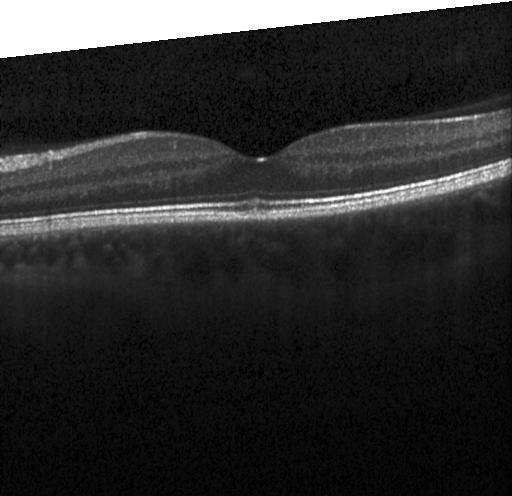

Horizontal scan through the fovea; optical coherence tomography B-scan
Finding: no CNV, DME, or drusen.